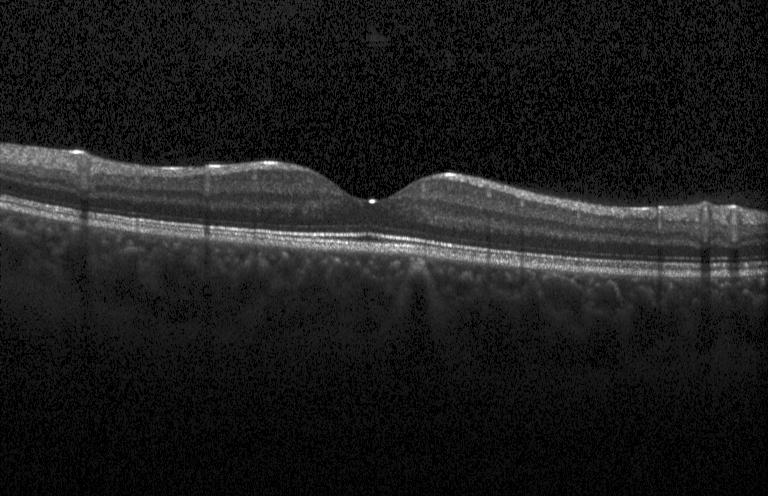

Retinal OCT cross-section
Macular OCT: no choroidal neovascularization, no diabetic macular edema, and no drusen.